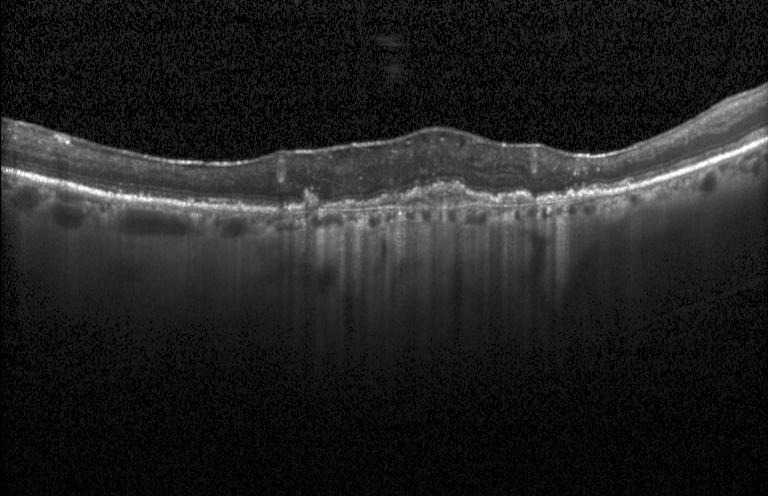

Diagnosis: choroidal neovascularization (CNV).